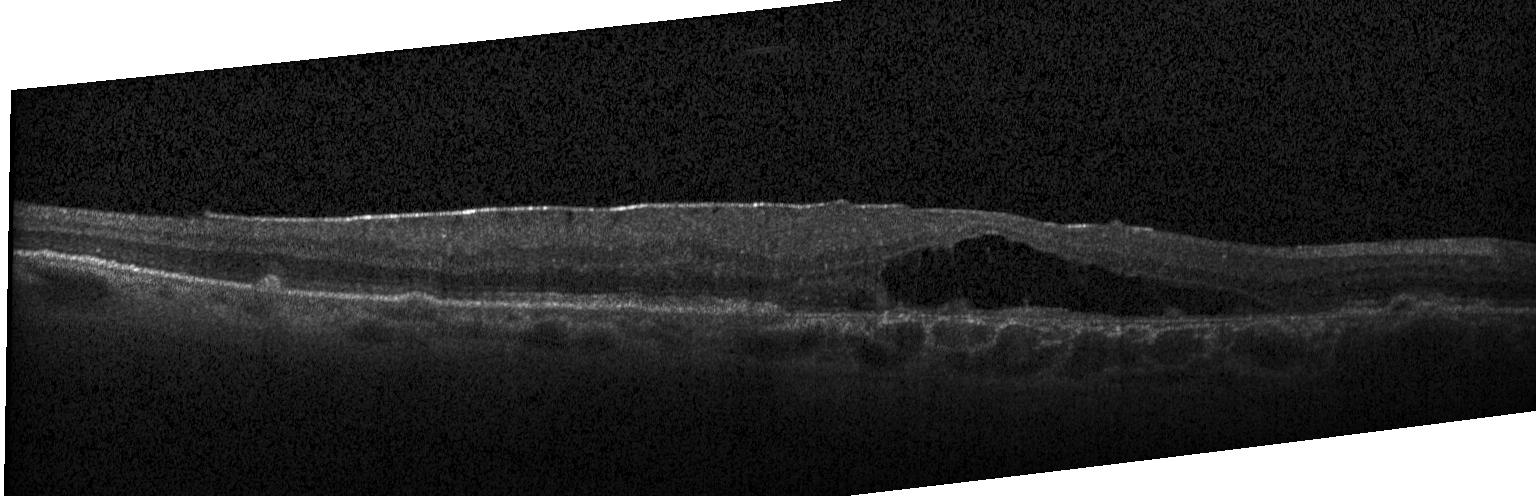 Diagnosis: choroidal neovascularization.